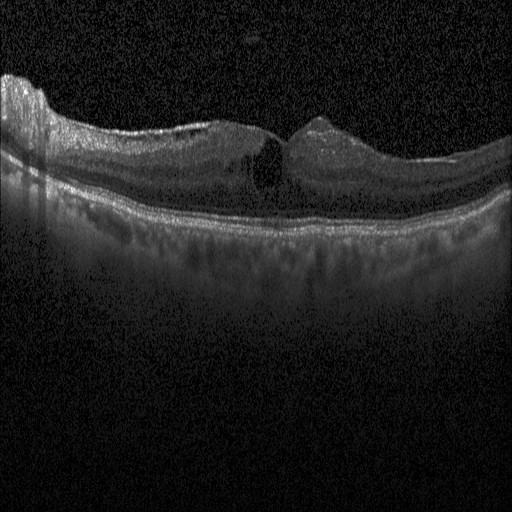

Instrument: Heidelberg Spectralis; optical coherence tomography scan; through the macula; SD-OCT — Impression: DME.